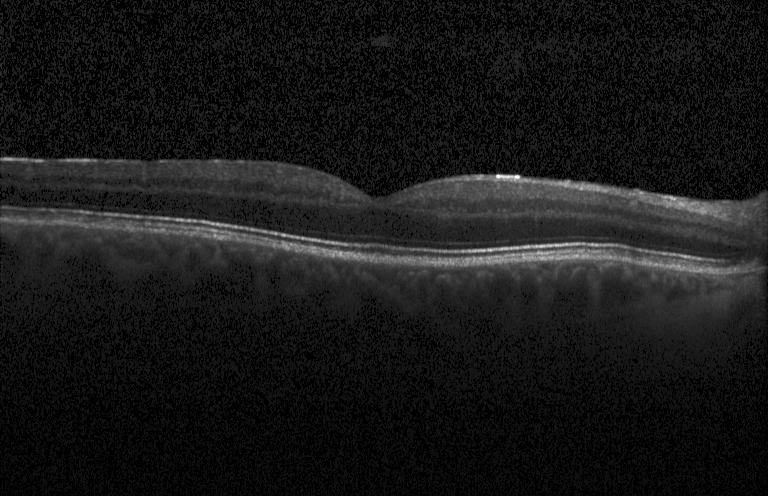
Optical coherence tomography B-scan.
No CNV, DME, or drusen.